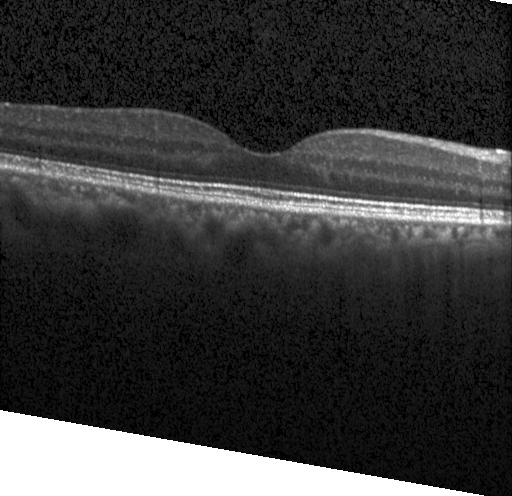 This B-scan demonstrates neither choroidal neovascularization, diabetic macular edema, nor drusen.